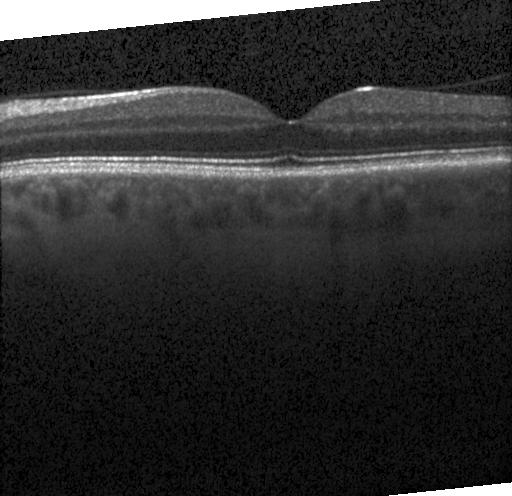

Optical coherence tomography B-scan. Heidelberg Spectralis OCT system
Finding: no choroidal neovascularization, no diabetic macular edema, and no drusen.